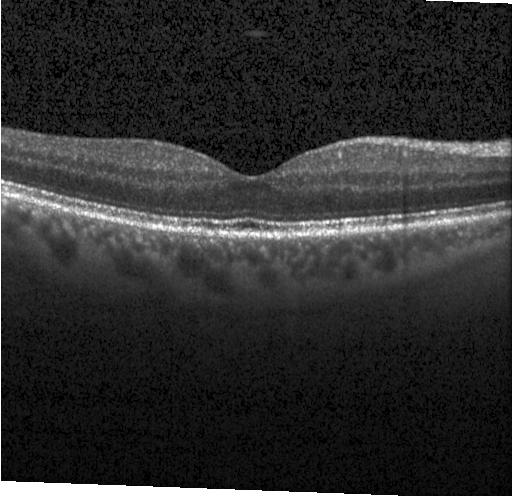

SD-OCT · acquired on a Heidelberg Spectralis · retinal OCT B-scan. Assessment: no evidence of choroidal neovascularization, diabetic macular edema, or drusen.